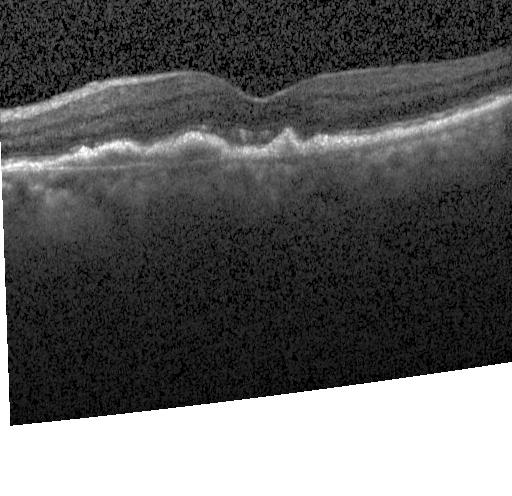

Finding: a choroidal neovascular membrane.